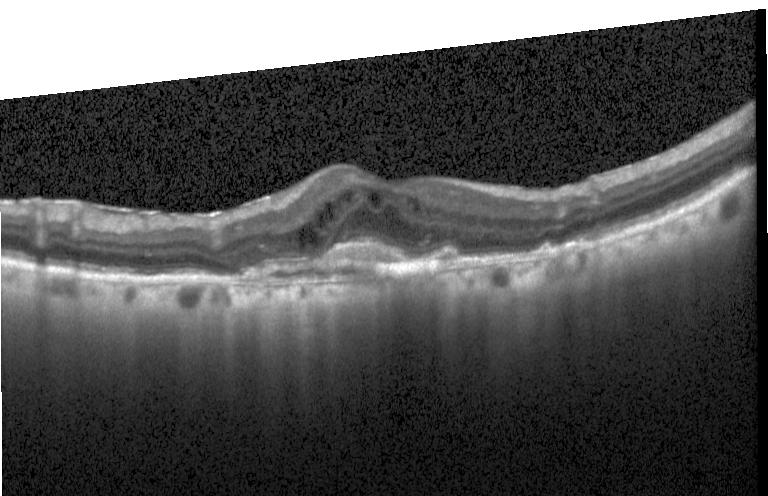 Spectral-domain OCT. Instrument: Heidelberg Spectralis. OCT B-scan — Macular OCT: a choroidal neovascular membrane.